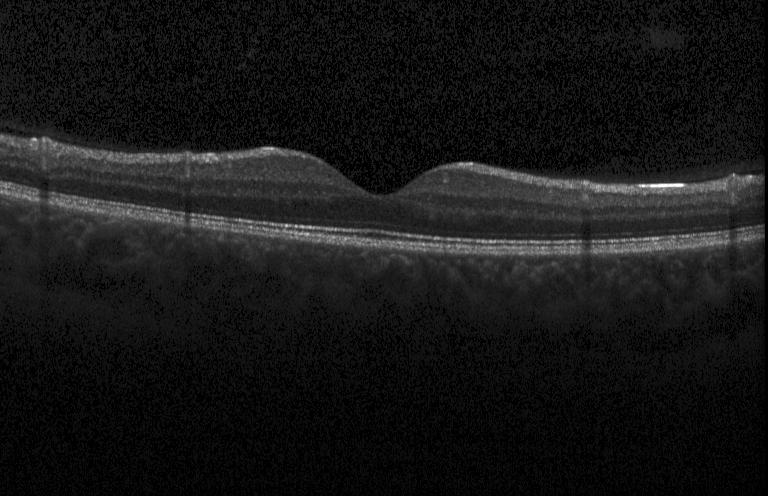 Macular OCT demonstrating no CNV, no DME, and no drusen.